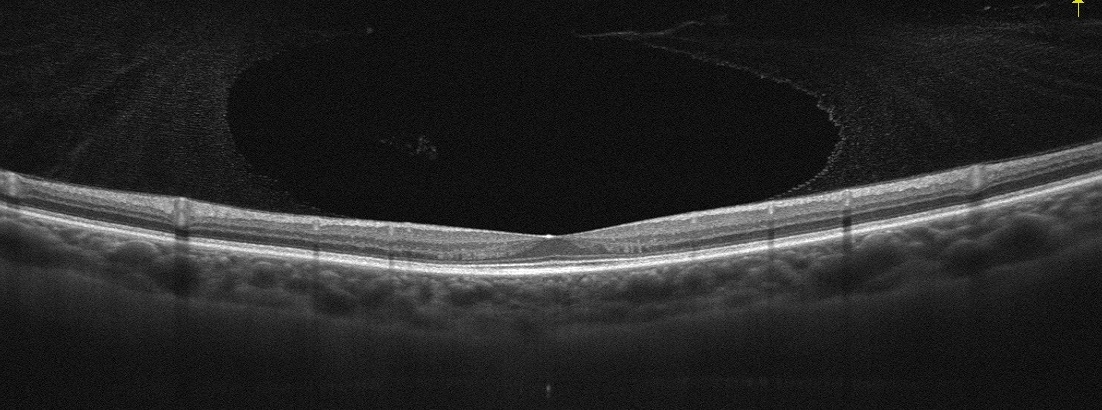 Retinal OCT cross-section; Optovue Avanti RTVue XR; fovea-centered
Diagnosis: absence of AMD, DME, ERM, RAO, RVO, and vitreomacular interface disease.